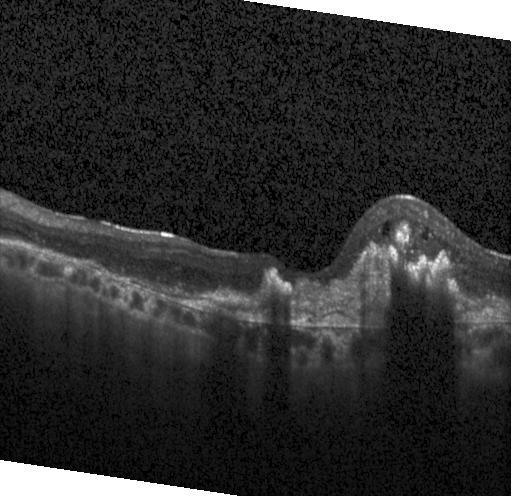
Assessment: a choroidal neovascular membrane.